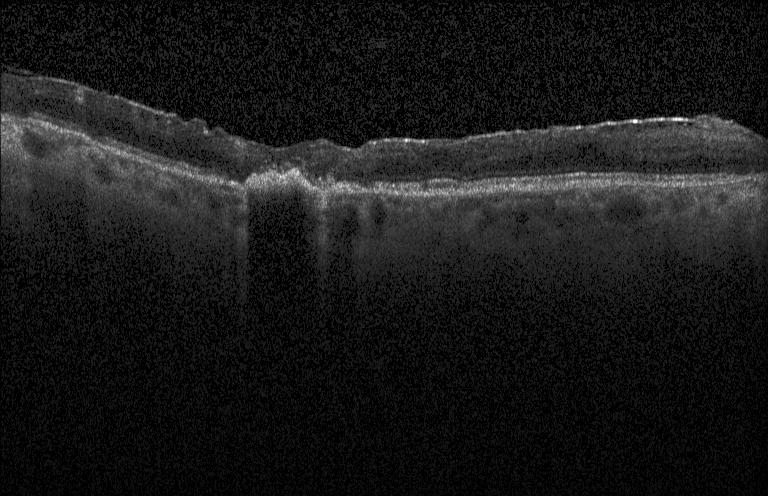
Retinal OCT B-scan, spectral-domain OCT, centered on the fovea. OCT finding: a choroidal neovascular membrane.